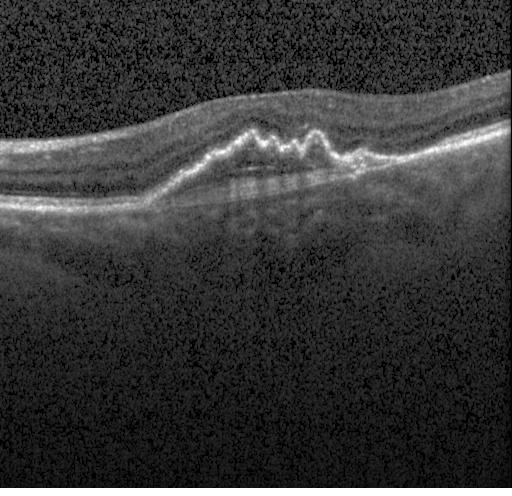 Finding: CNV.